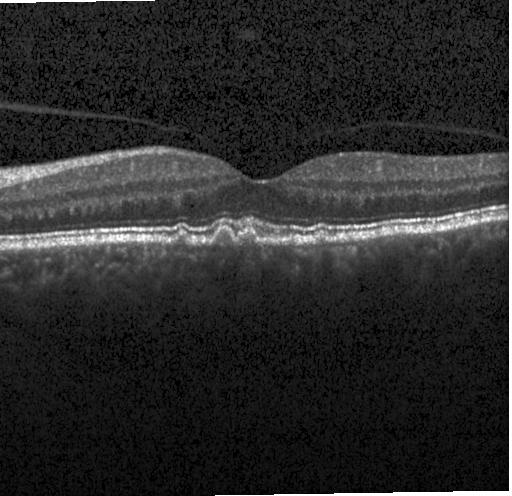
Retinal OCT cross-section — Impression: sub-RPE drusenoid deposits.